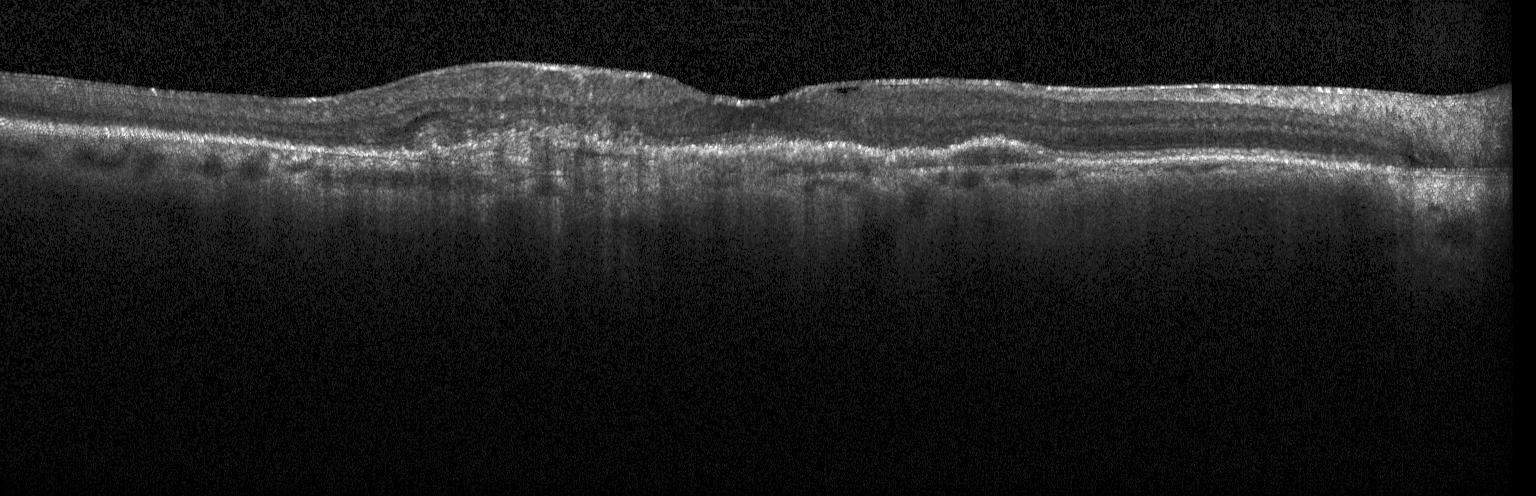
Optical coherence tomography scan · SD-OCT. Impression: a choroidal neovascular membrane.